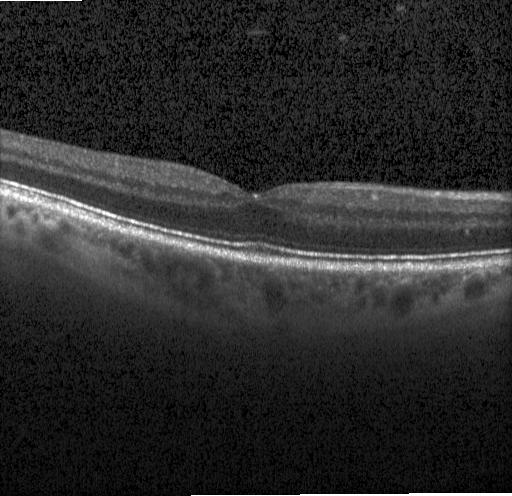 Dx: no evidence of choroidal neovascularization, diabetic macular edema, or drusen.